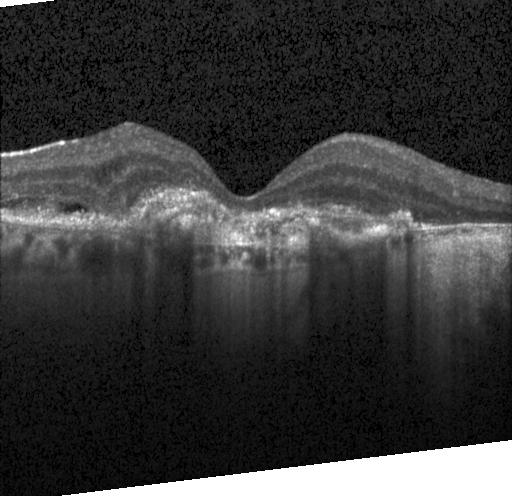

Heidelberg Spectralis, SD-OCT, macular scan, OCT line scan.
Impression: a choroidal neovascular membrane.